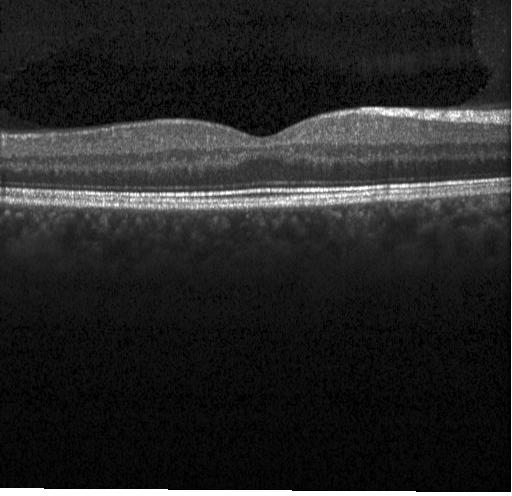

Impression: neither choroidal neovascularization, diabetic macular edema, nor drusen.